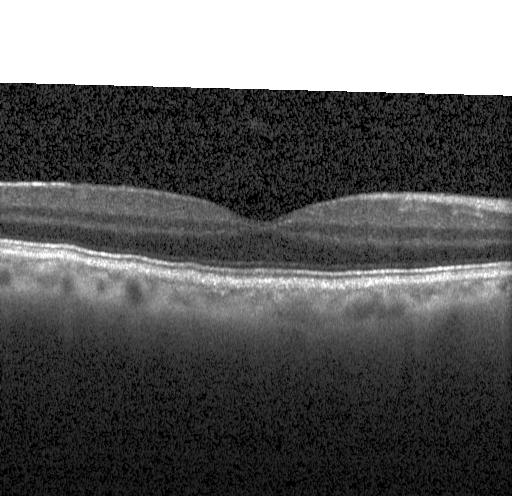
OCT B-scan showing no evidence of CNV, DME, or drusen.